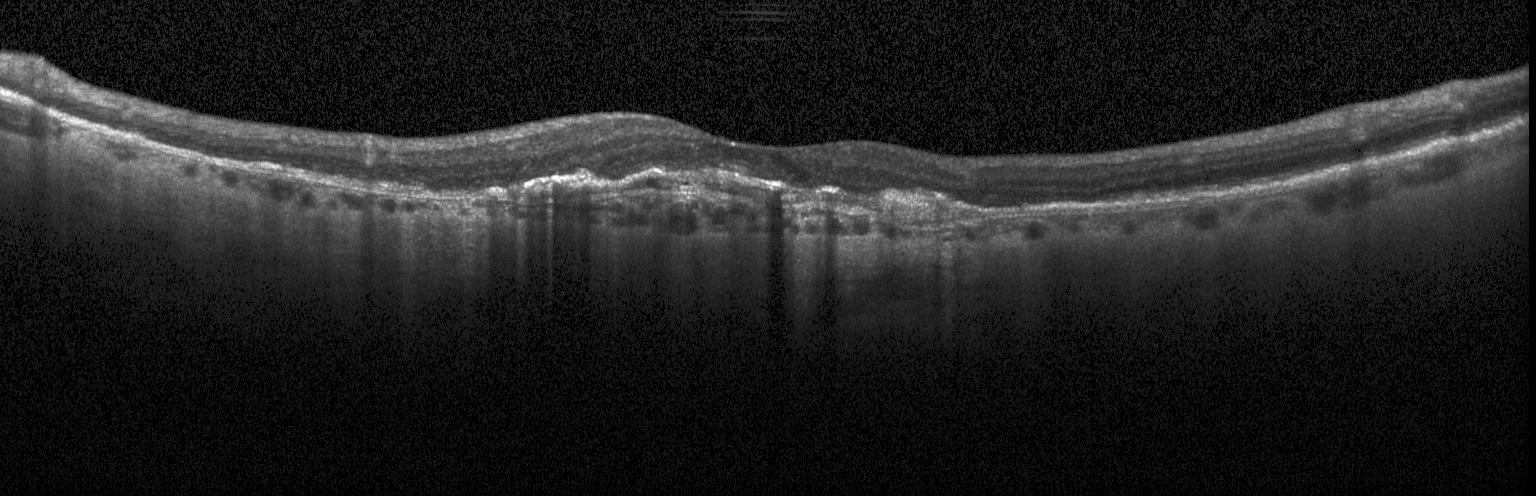 Macular OCT demonstrating a choroidal neovascular membrane.